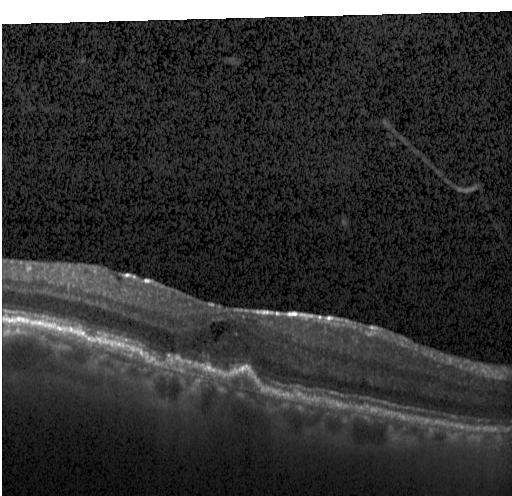 OCT line scan.
This B-scan demonstrates CNV.